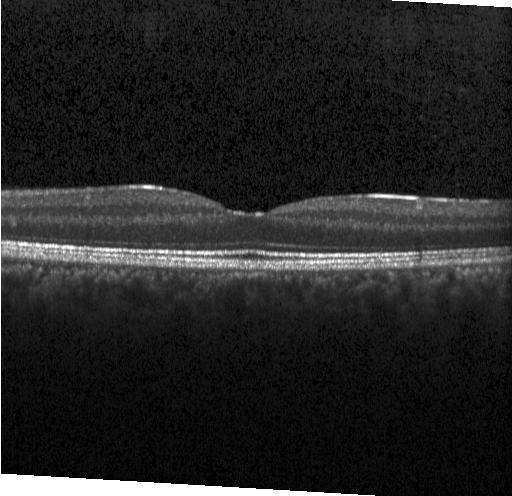 Finding: neither CNV, DME, nor drusen.